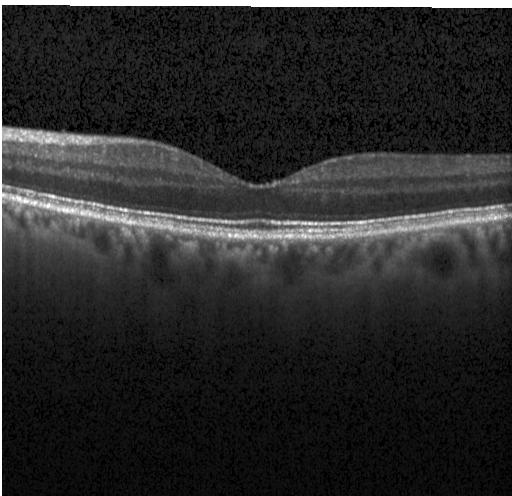
Dx: no CNV, no DME, and no drusen.